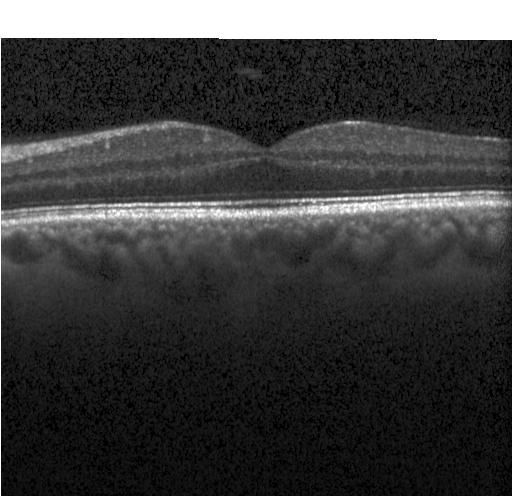
Retinal OCT cross-section
This B-scan demonstrates neither CNV, DME, nor drusen.